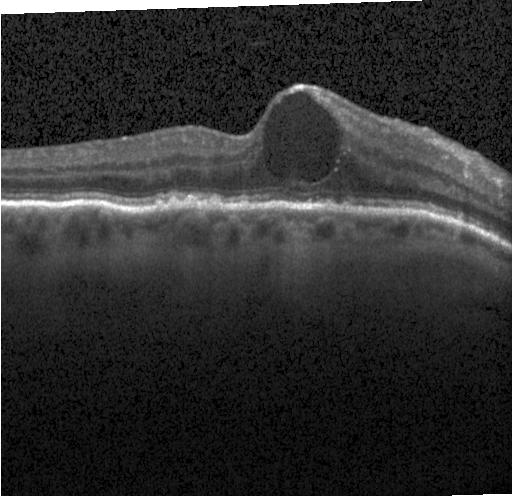
Finding: choroidal neovascularization (CNV).